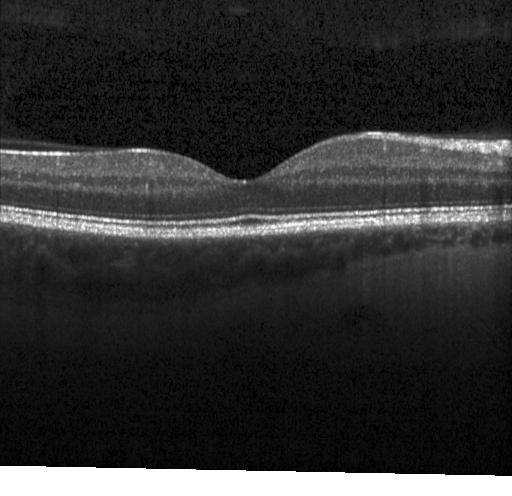
Through the macula, retinal OCT B-scan. OCT finding: no choroidal neovascularization, no diabetic macular edema, and no drusen.